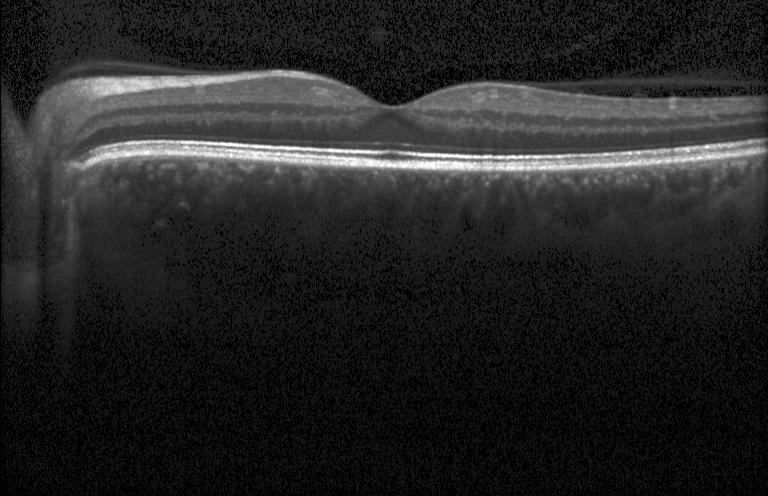

Diagnosis: no evidence of choroidal neovascularization, diabetic macular edema, or drusen.